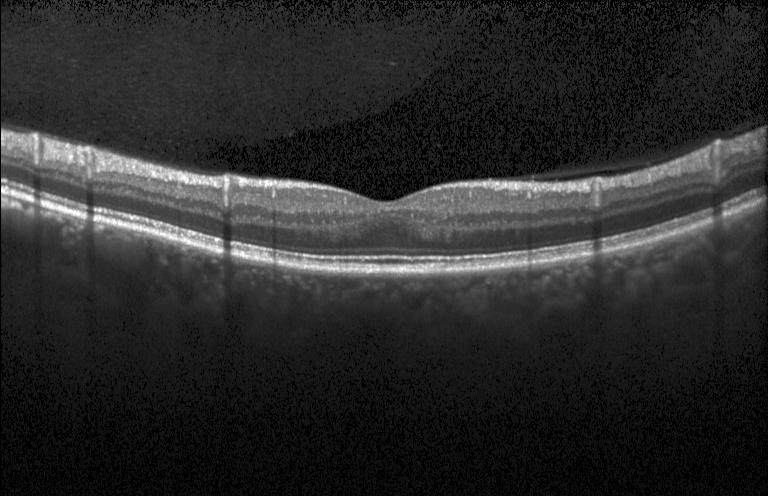
Impression: neither CNV, DME, nor drusen.